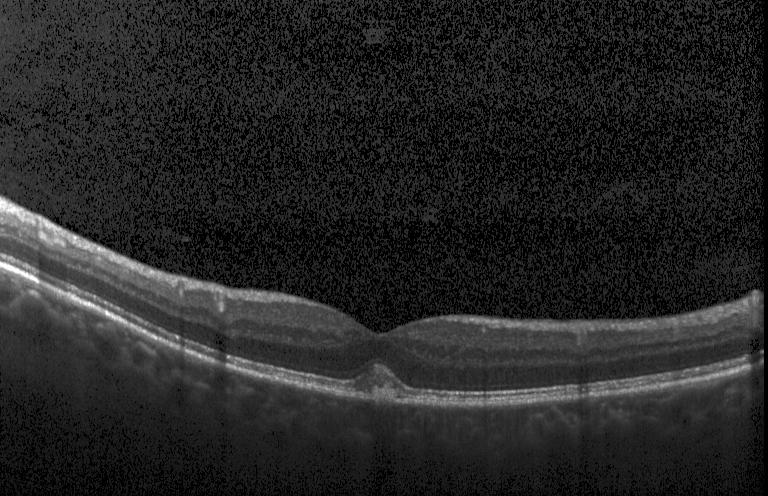
Dx: sub-RPE drusenoid deposits.